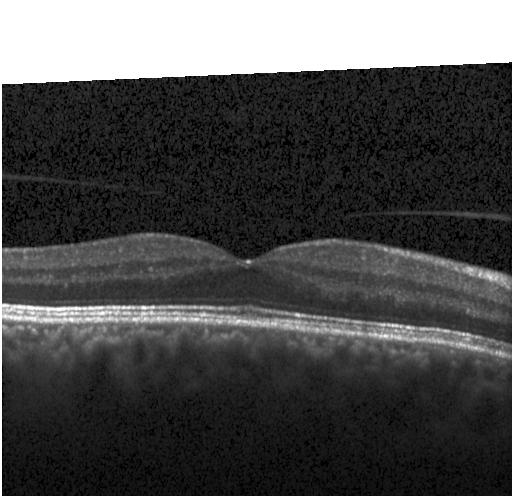

Finding: no evidence of choroidal neovascularization, diabetic macular edema, or drusen.